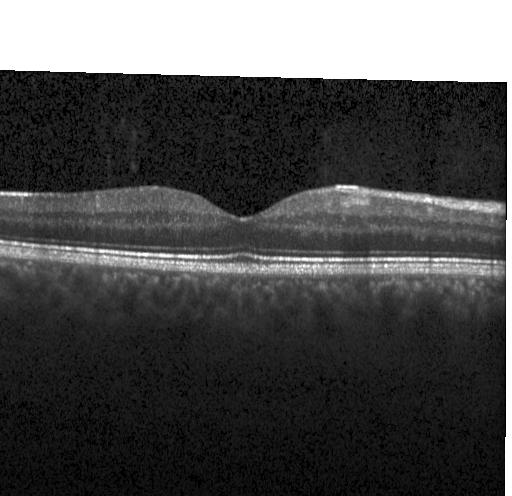

Centered on the fovea, retinal OCT cross-section, spectral-domain OCT, Heidelberg Spectralis OCT system.
Neither choroidal neovascularization, diabetic macular edema, nor drusen.